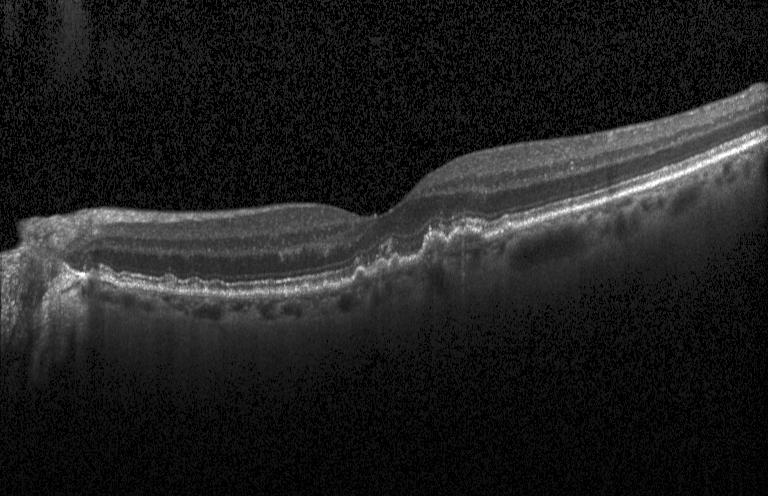 OCT line scan
Diagnosis: CNV.